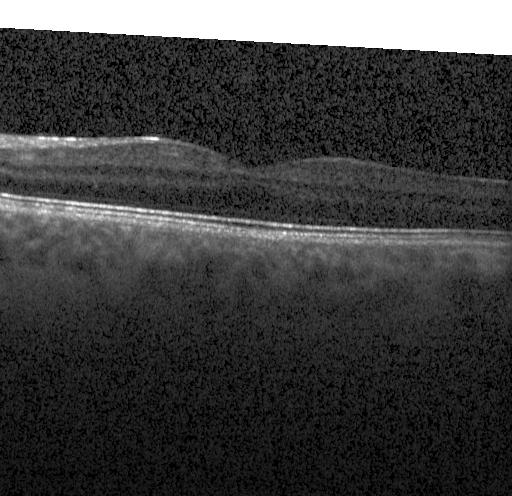 Optical coherence tomography scan
The scan shows no choroidal neovascularization, no diabetic macular edema, and no drusen.